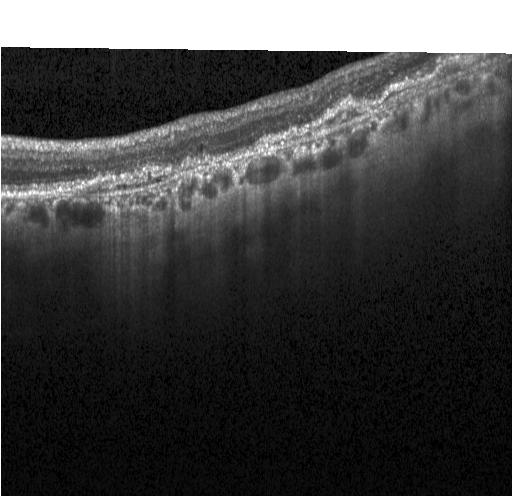

Through the macula. Optical coherence tomography B-scan — Finding: a choroidal neovascular membrane.